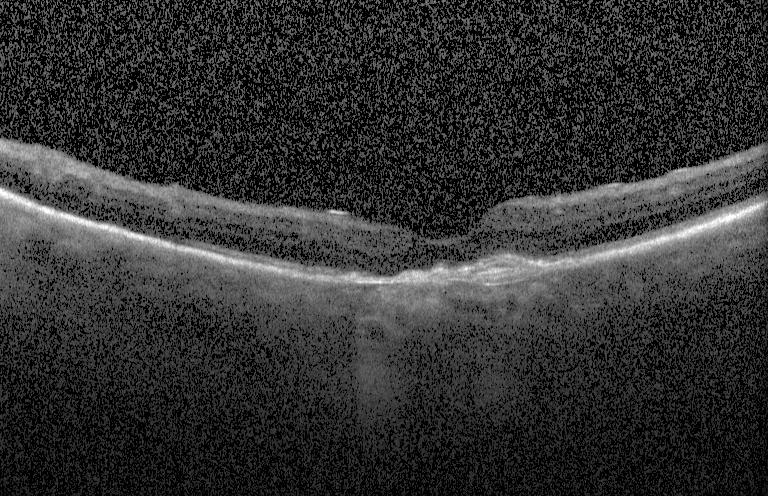 Dx: a choroidal neovascular membrane.